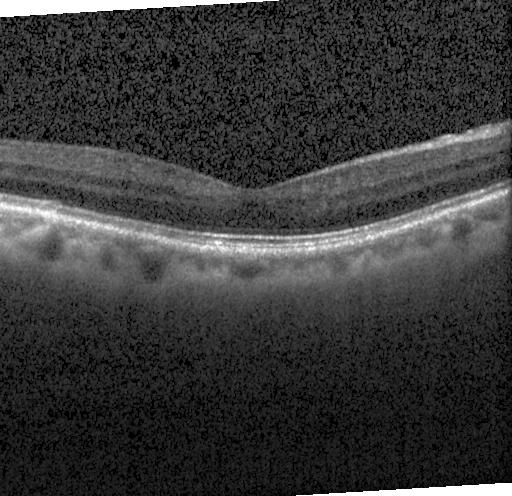

Fovea-centered. Optical coherence tomography B-scan.
Macular OCT: neither choroidal neovascularization, diabetic macular edema, nor drusen.